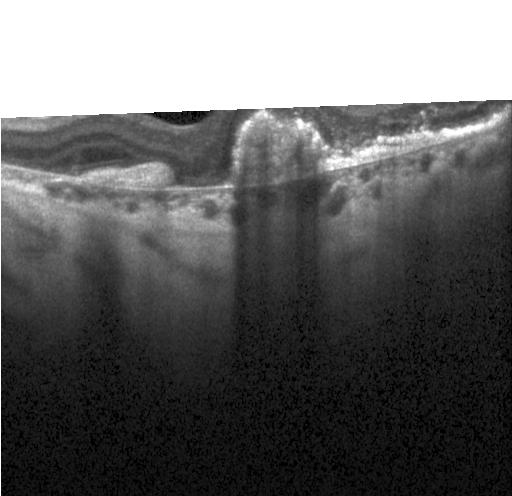

OCT B-scan; spectral-domain optical coherence tomography — Impression: choroidal neovascularization (CNV).